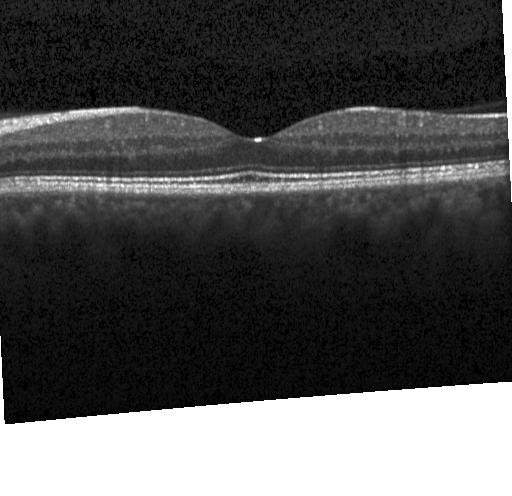

OCT finding: no choroidal neovascularization, no diabetic macular edema, and no drusen.